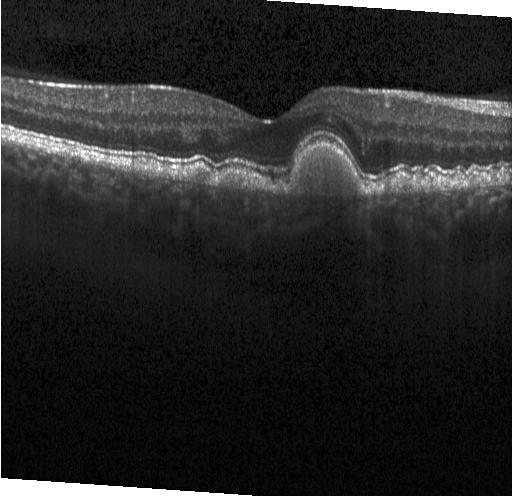

Fovea-centered · retinal OCT B-scan.
The scan shows multiple drusen.